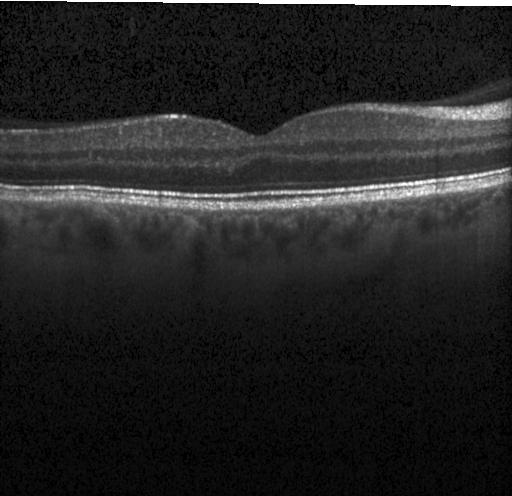
Spectral-domain optical coherence tomography, Heidelberg Spectralis OCT system, optical coherence tomography B-scan.
Dx: no evidence of choroidal neovascularization, diabetic macular edema, or drusen.